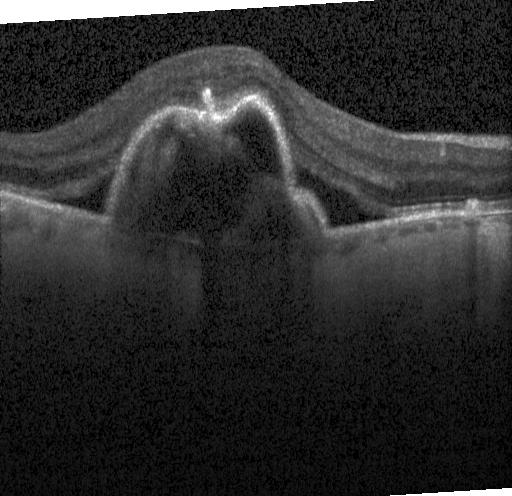 OCT B-scan; spectral-domain OCT; centered on the fovea
OCT finding: CNV.